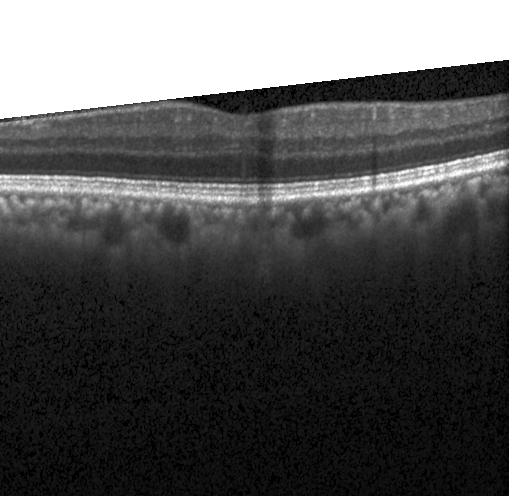 Macular OCT demonstrating no evidence of choroidal neovascularization, diabetic macular edema, or drusen.